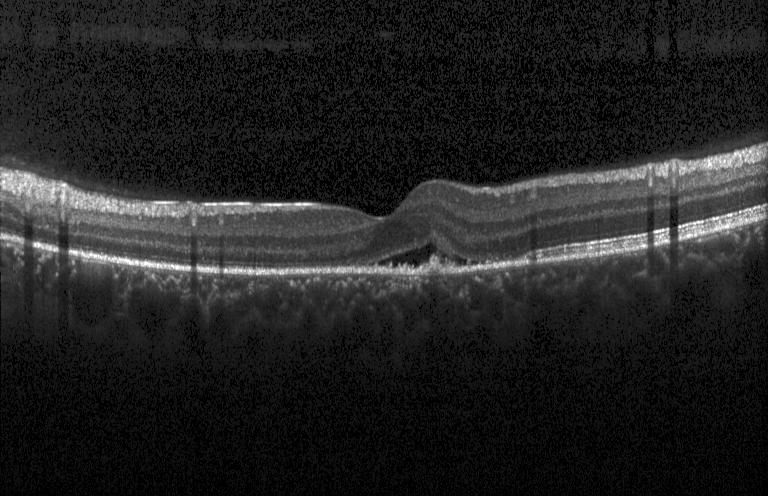
SD-OCT. OCT B-scan. Horizontal scan through the fovea. Dx: choroidal neovascularization (CNV).